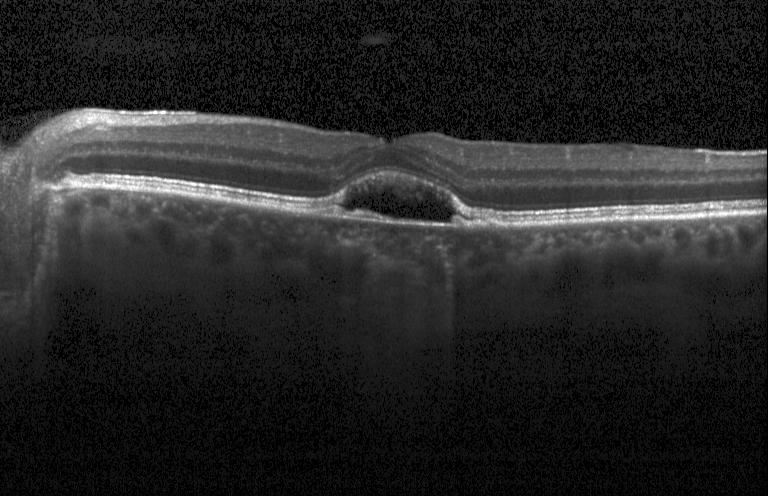 OCT B-scan; acquired on a Heidelberg Spectralis; fovea-centered.
OCT finding: a choroidal neovascular membrane.